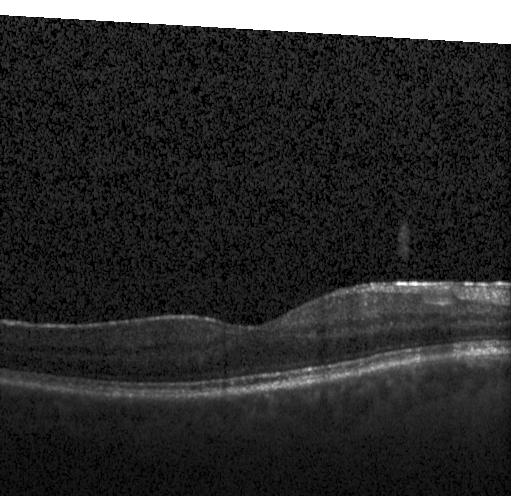

OCT B-scan; Heidelberg Spectralis — Impression: neither choroidal neovascularization, diabetic macular edema, nor drusen.